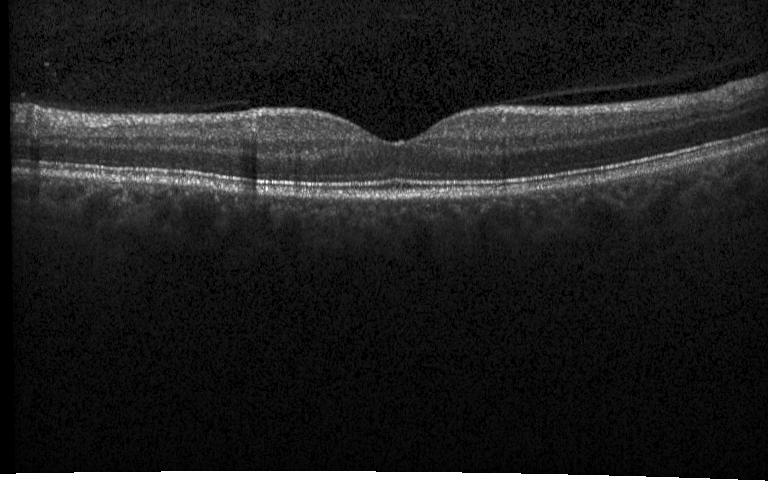

OCT scan showing no evidence of choroidal neovascularization, diabetic macular edema, or drusen.